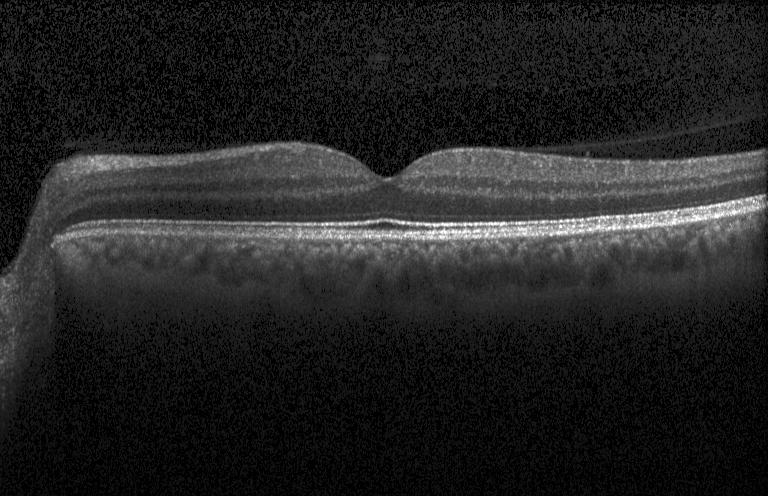
Spectral-domain OCT; optical coherence tomography B-scan
Impression: no CNV, no DME, and no drusen.